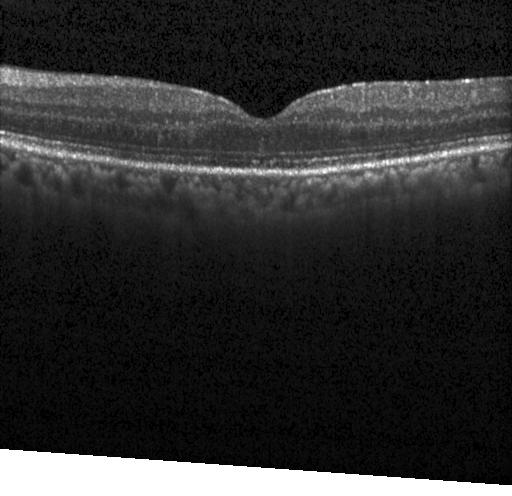

Optical coherence tomography B-scan. Finding: neither choroidal neovascularization, diabetic macular edema, nor drusen.